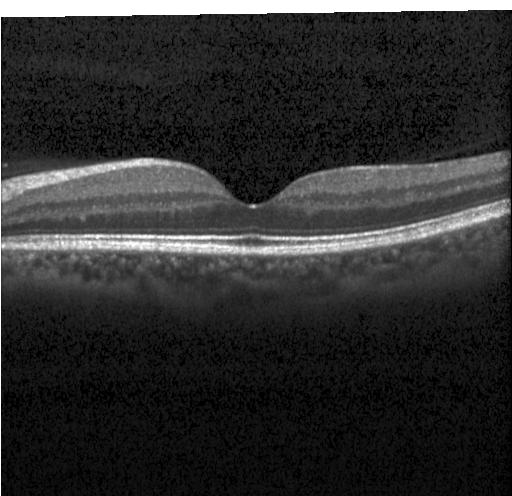

Retinal OCT B-scan — No evidence of choroidal neovascularization, diabetic macular edema, or drusen.